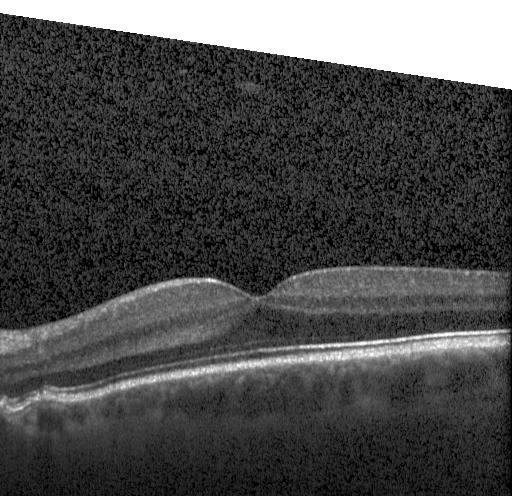 Horizontal scan through the fovea; acquired on a Heidelberg Spectralis; optical coherence tomography scan; spectral-domain optical coherence tomography
Assessment: sub-RPE drusenoid deposits.